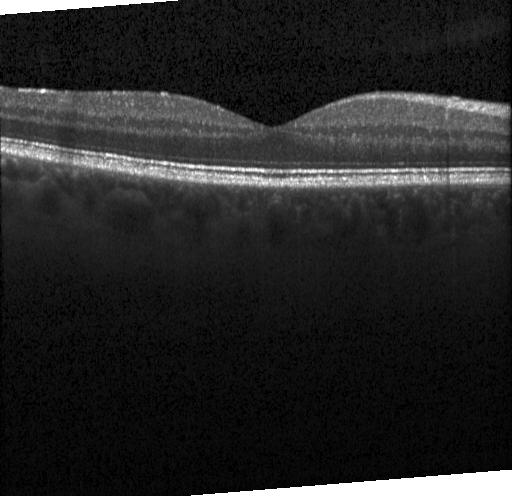 Spectral-domain OCT B-scan: no evidence of CNV, DME, or drusen.